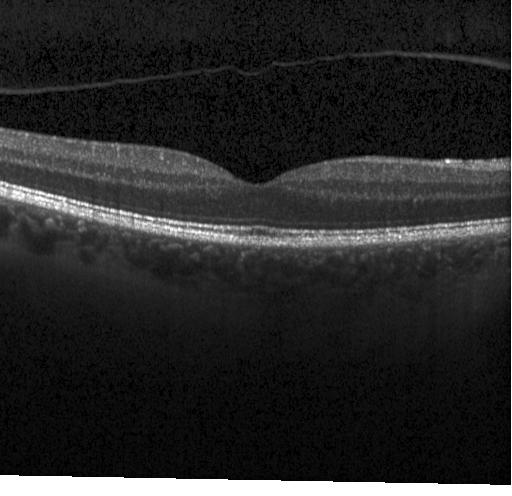
OCT line scan
Dx: neither choroidal neovascularization, diabetic macular edema, nor drusen.